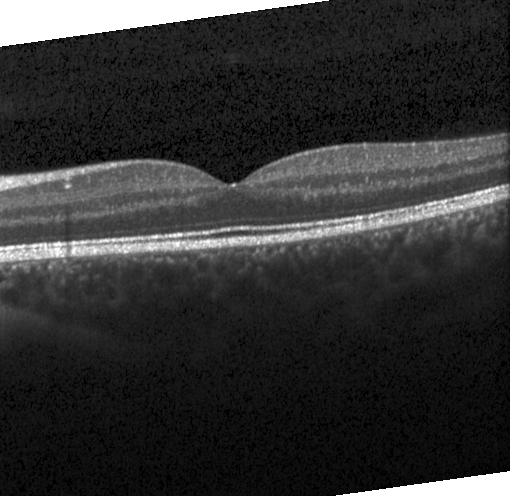 Acquired on a Heidelberg Spectralis · retinal OCT B-scan · fovea-centered — Finding: no evidence of CNV, DME, or drusen.